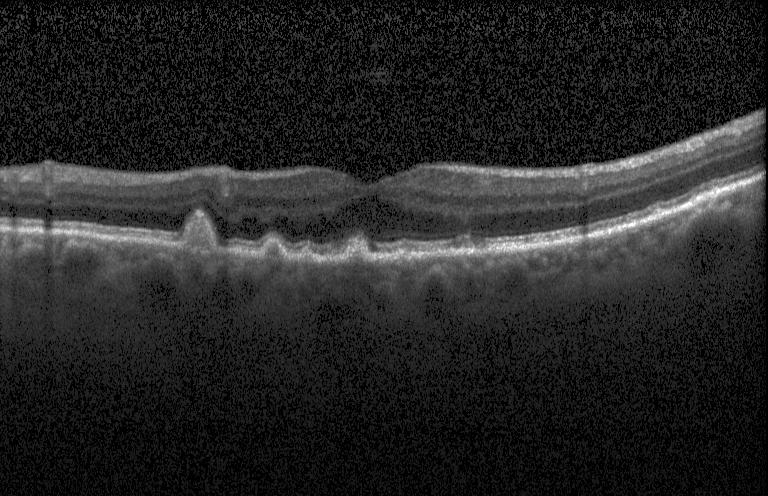
SD-OCT. Retinal OCT B-scan
Finding: multiple drusen.